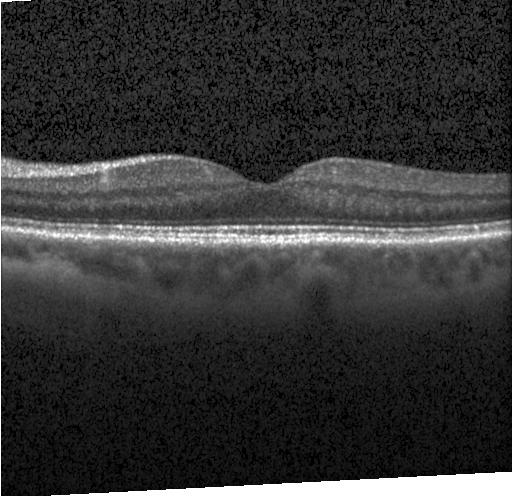
OCT scan showing neither CNV, DME, nor drusen.